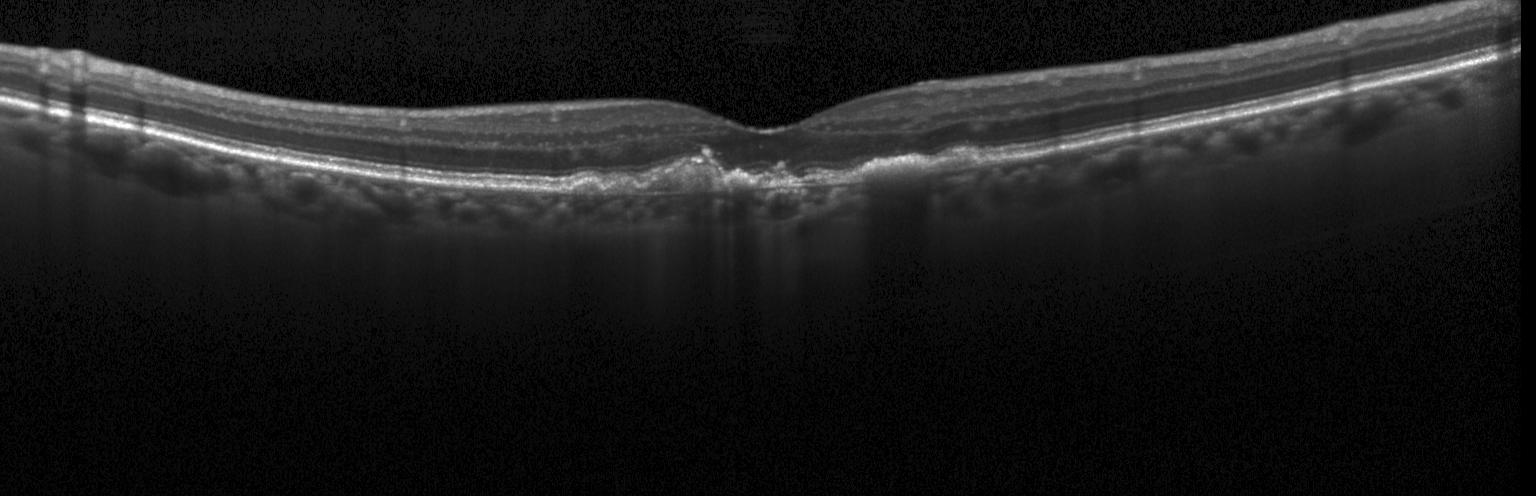

Impression: sub-RPE drusenoid deposits.